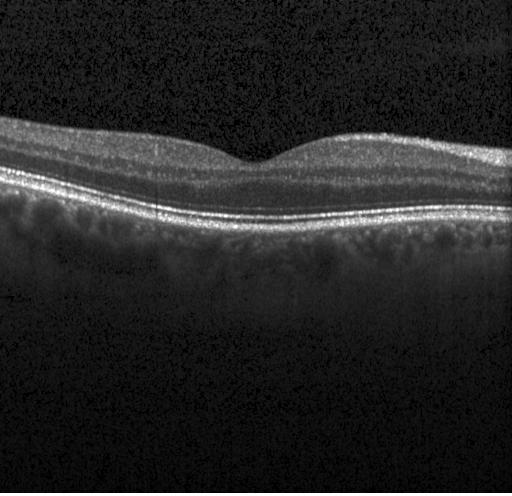 SD-OCT; retinal OCT B-scan; acquired on a Heidelberg Spectralis; centered on the fovea.
No evidence of choroidal neovascularization, diabetic macular edema, or drusen.